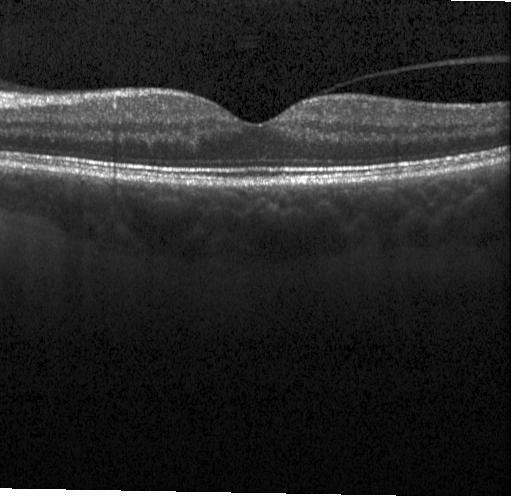 Retinal OCT cross-section; instrument: Heidelberg Spectralis
Neither choroidal neovascularization, diabetic macular edema, nor drusen.